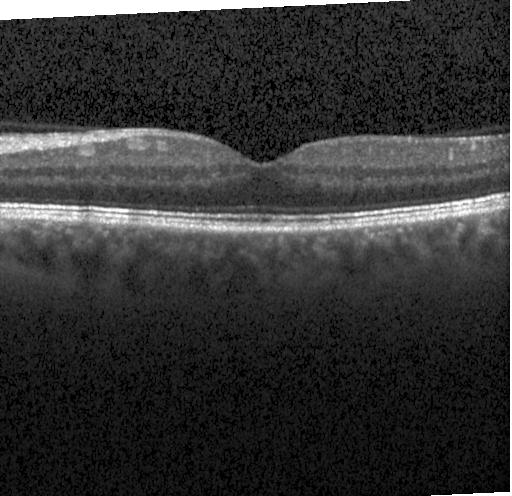

Horizontal scan through the fovea. Spectral-domain optical coherence tomography. Optical coherence tomography scan — Dx: no evidence of CNV, DME, or drusen.